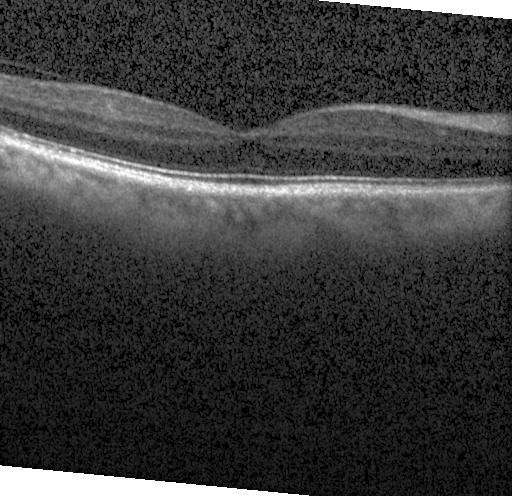 OCT B-scan · spectral-domain OCT · through the macula — Impression: no choroidal neovascularization, diabetic macular edema, or drusen.